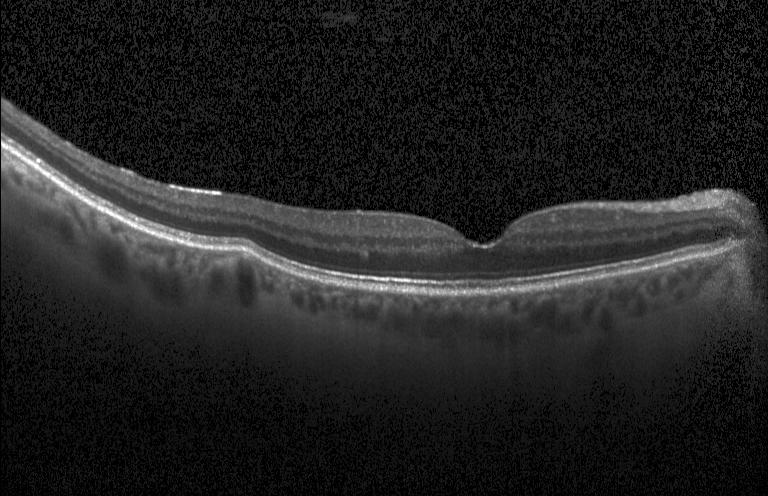
Finding: no choroidal neovascularization, no diabetic macular edema, and no drusen.